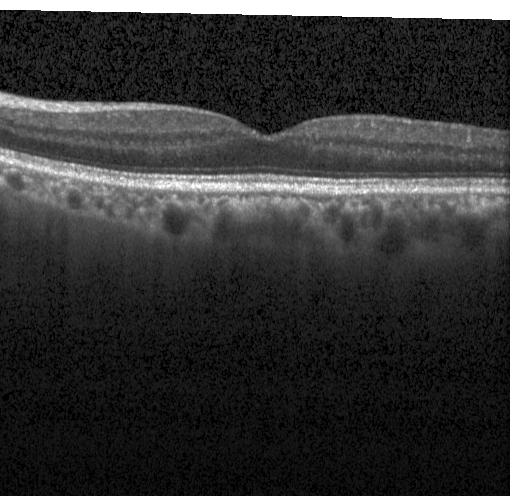
Optical coherence tomography scan. Heidelberg Spectralis OCT system
Impression: no choroidal neovascularization, no diabetic macular edema, and no drusen.